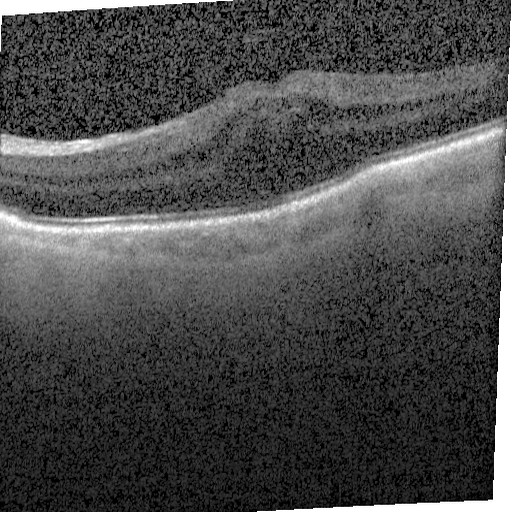
Retinal OCT cross-section; centered on the fovea; instrument: Heidelberg Spectralis; spectral-domain OCT. DME.